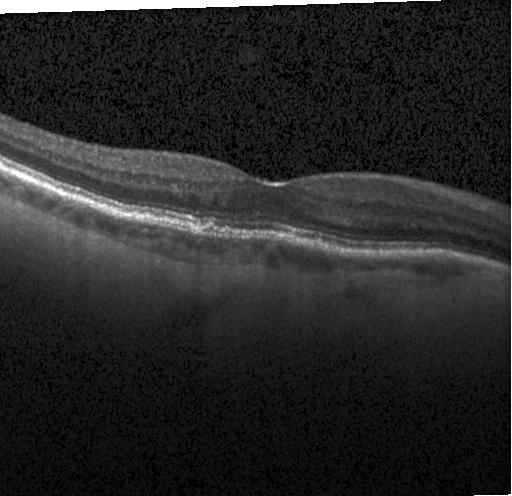 This B-scan demonstrates sub-RPE drusenoid deposits.